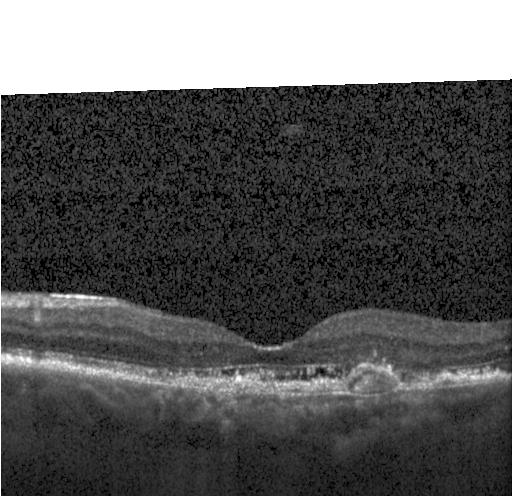 Dx: choroidal neovascularization.